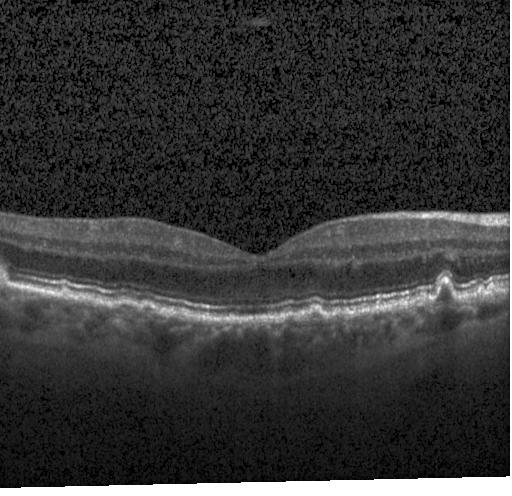 Retinal OCT B-scan · instrument: Heidelberg Spectralis — The scan shows multiple drusen.